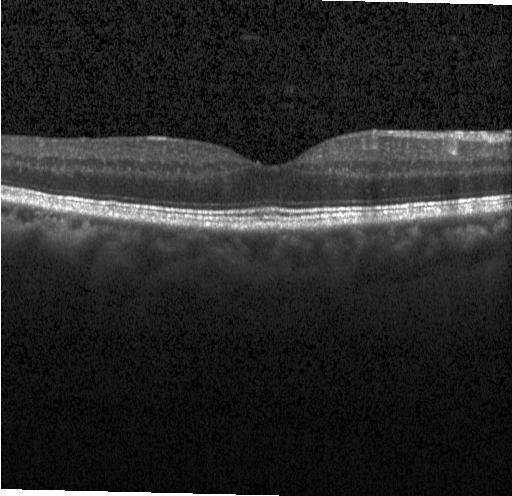 OCT scan showing no evidence of choroidal neovascularization, diabetic macular edema, or drusen.